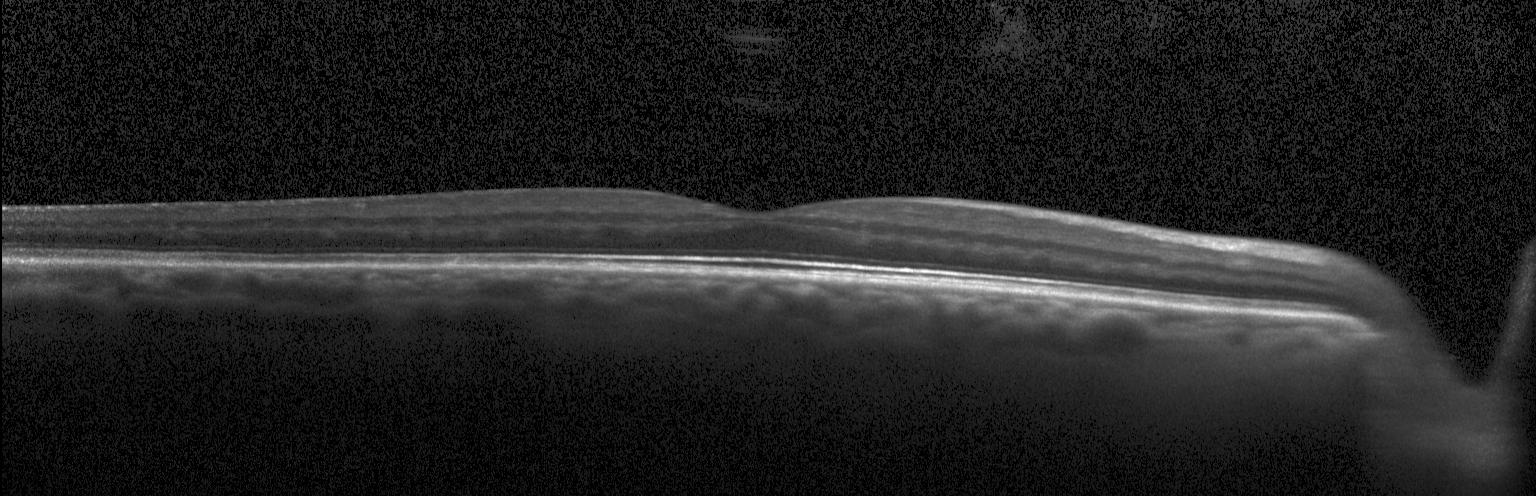 Fovea-centered; OCT line scan; Heidelberg Spectralis; spectral-domain optical coherence tomography. Diagnosis: no evidence of choroidal neovascularization, diabetic macular edema, or drusen.